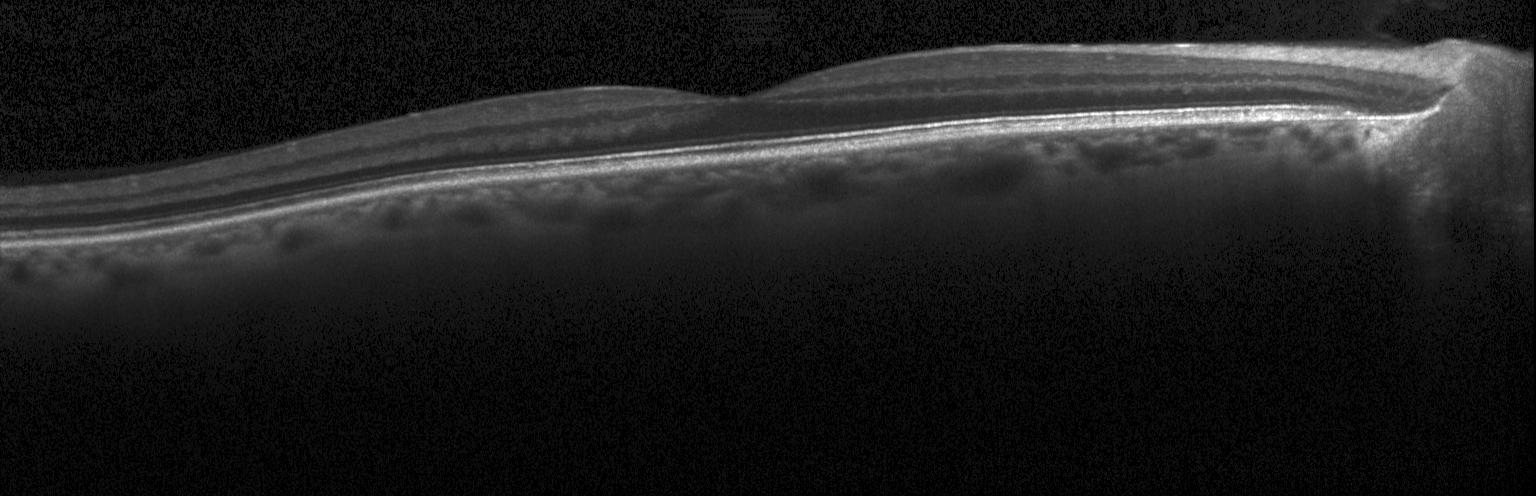

Macular scan. Heidelberg Spectralis. OCT line scan.
Diagnosis: no evidence of choroidal neovascularization, diabetic macular edema, or drusen.